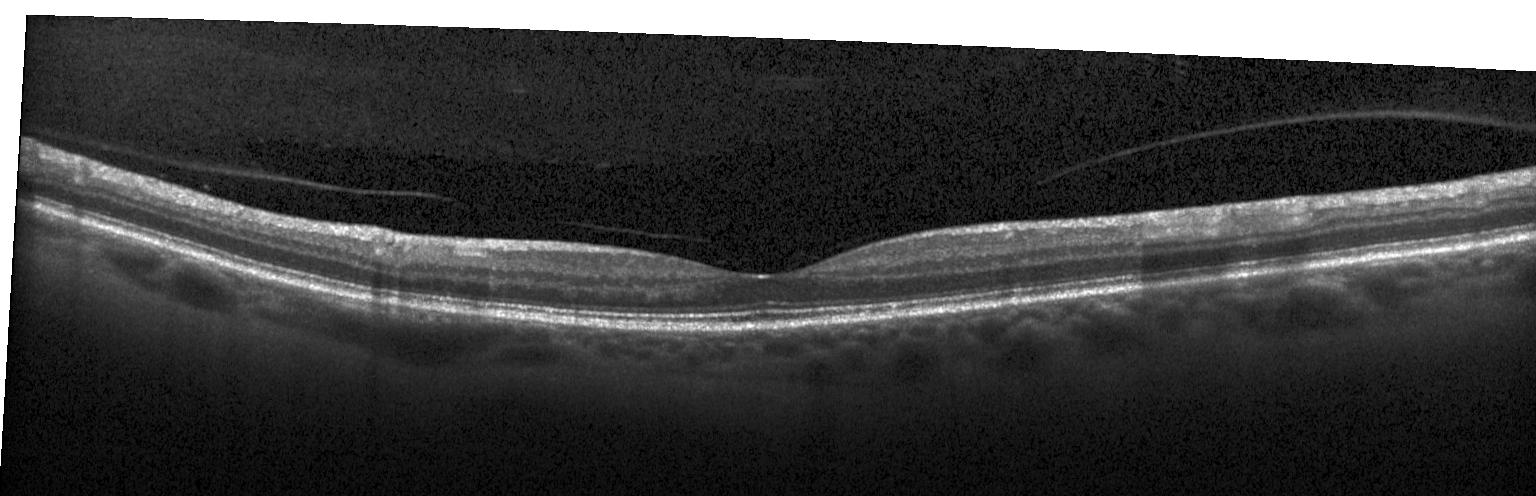
Instrument: Heidelberg Spectralis · retinal OCT B-scan — The scan shows neither choroidal neovascularization, diabetic macular edema, nor drusen.